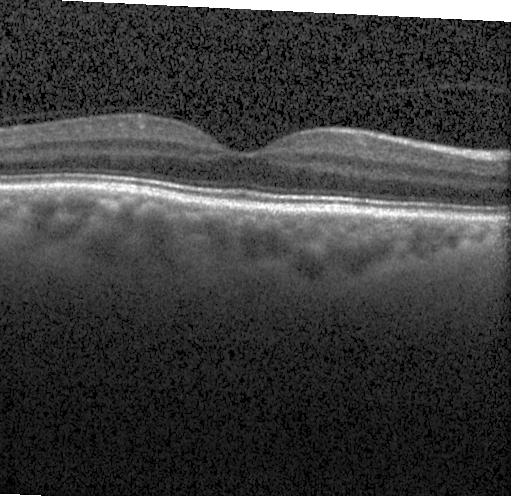

Diagnosis: no evidence of choroidal neovascularization, diabetic macular edema, or drusen.